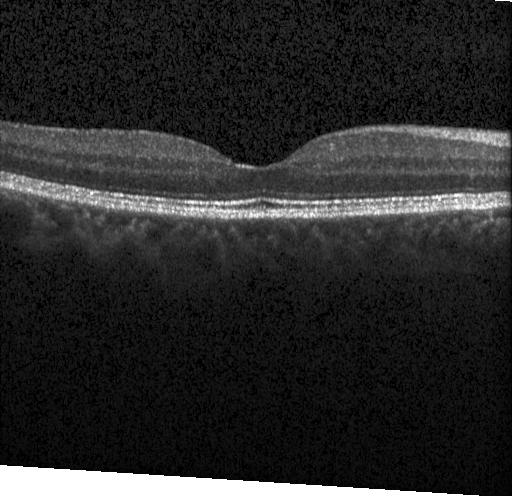

Spectral-domain optical coherence tomography. Retinal OCT B-scan. Centered on the fovea. Heidelberg Spectralis
This B-scan demonstrates no choroidal neovascularization, diabetic macular edema, or drusen.